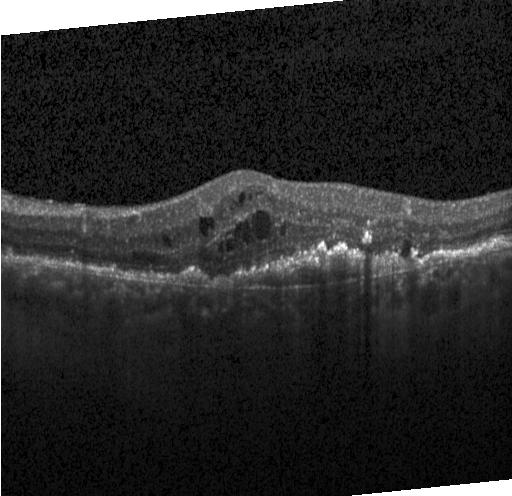 Spectral-domain OCT, OCT B-scan.
Macular OCT: choroidal neovascularization (CNV).